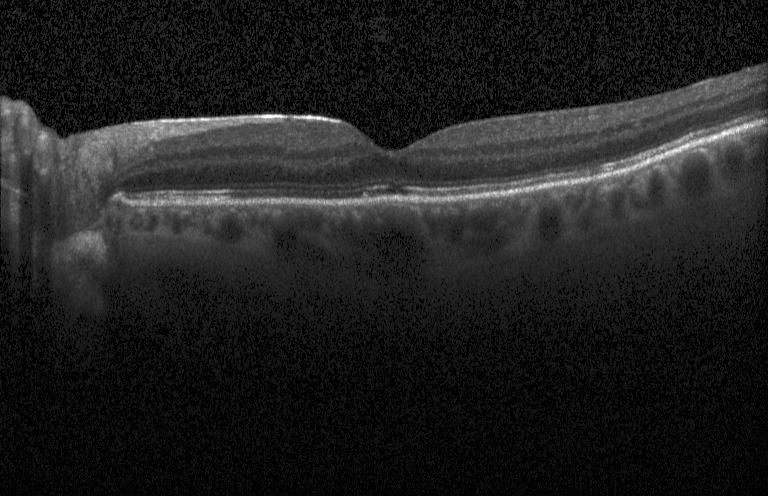 Retinal OCT B-scan. This B-scan demonstrates no evidence of choroidal neovascularization, diabetic macular edema, or drusen.